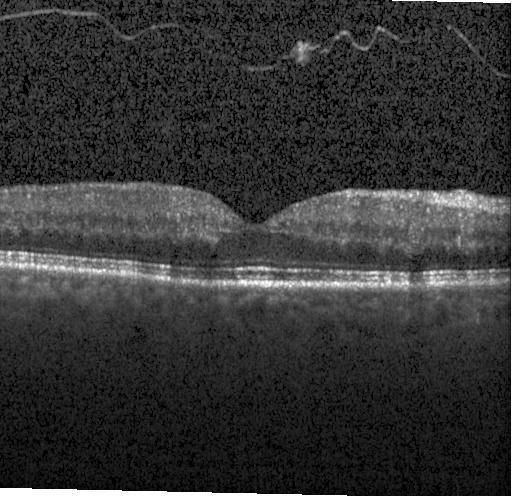 OCT scan showing neither CNV, DME, nor drusen.